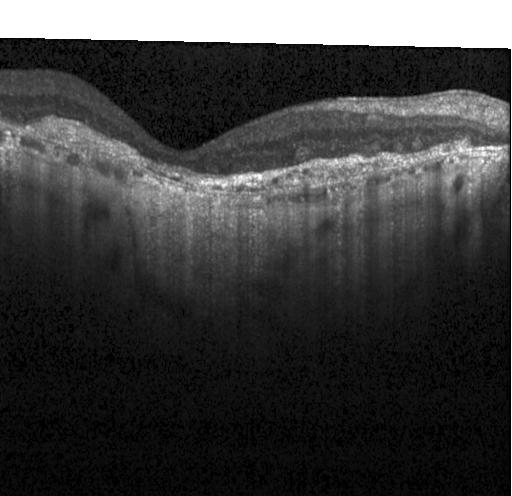
Retinal OCT cross-section.
Impression: a choroidal neovascular membrane.